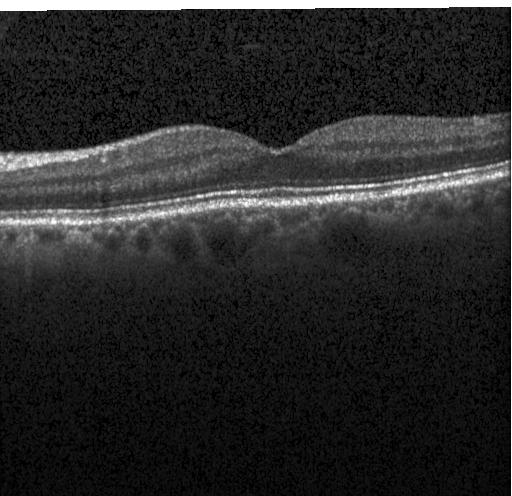
Spectral-domain optical coherence tomography, horizontal scan through the fovea, OCT B-scan, Heidelberg Spectralis OCT system — OCT finding: no choroidal neovascularization, no diabetic macular edema, and no drusen.